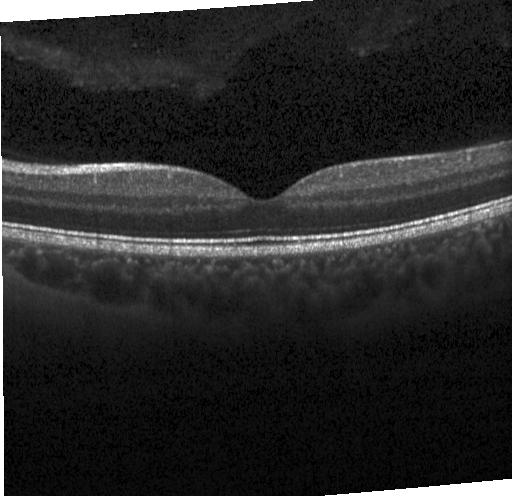
OCT B-scan
Finding: no CNV, no DME, and no drusen.